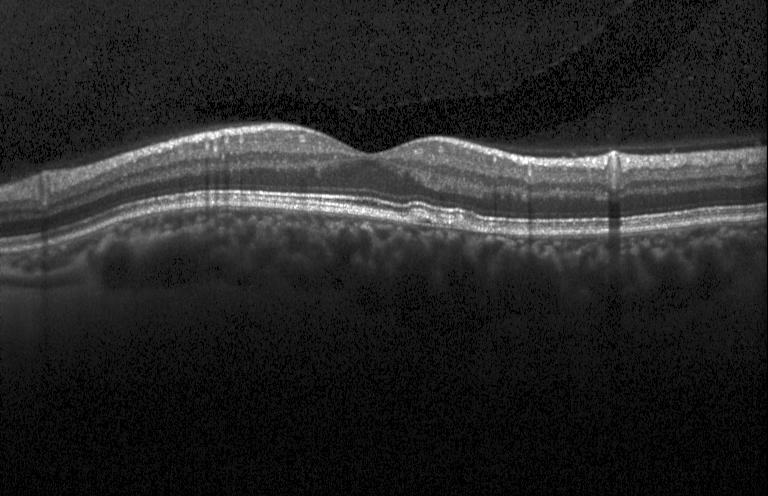

Finding: a choroidal neovascular membrane.